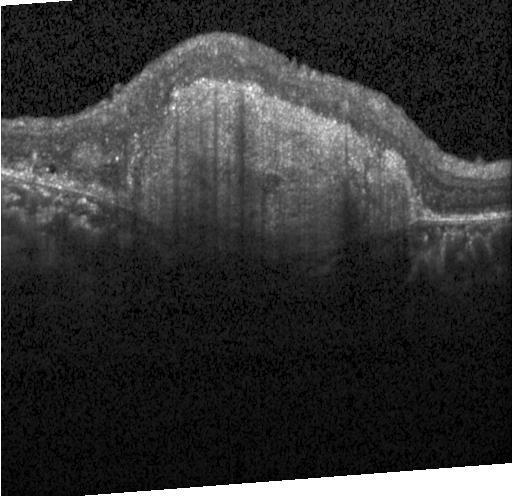

This B-scan demonstrates a choroidal neovascular membrane.